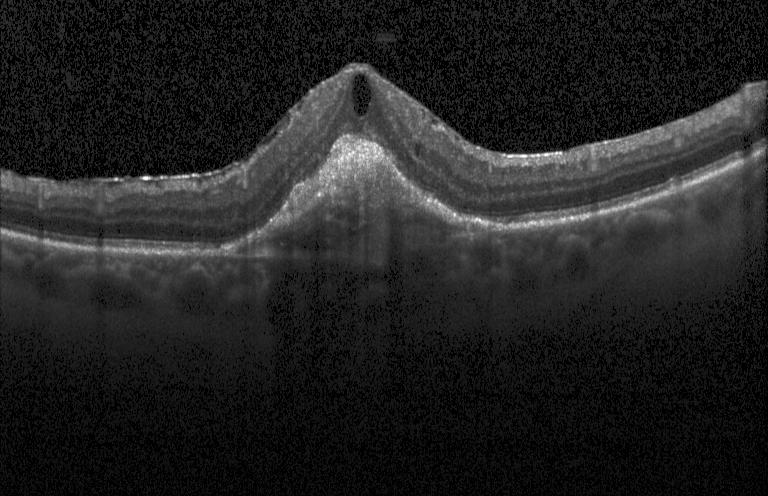

Horizontal scan through the fovea. Optical coherence tomography scan.
Diagnosis: a choroidal neovascular membrane.